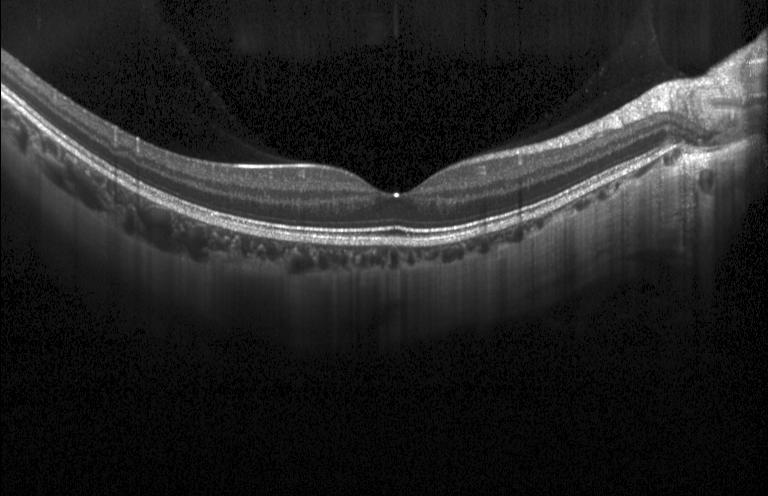 Optical coherence tomography scan.
No evidence of CNV, DME, or drusen.